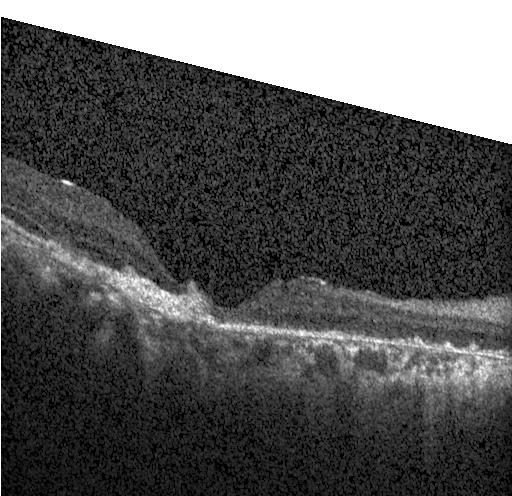
Assessment: choroidal neovascularization.